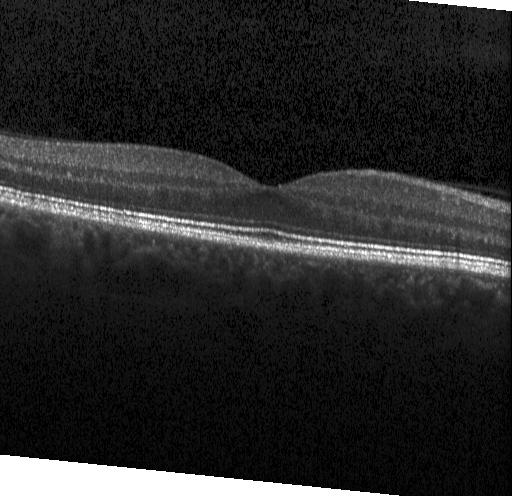 Acquired on a Heidelberg Spectralis. OCT line scan. Finding: no CNV, DME, or drusen.